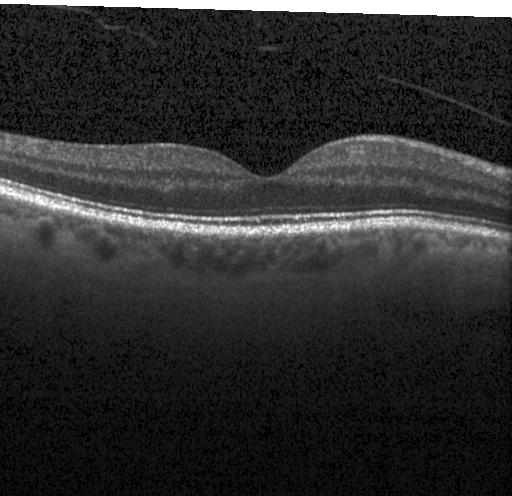 Spectral-domain optical coherence tomography · OCT line scan.
Finding: neither CNV, DME, nor drusen.